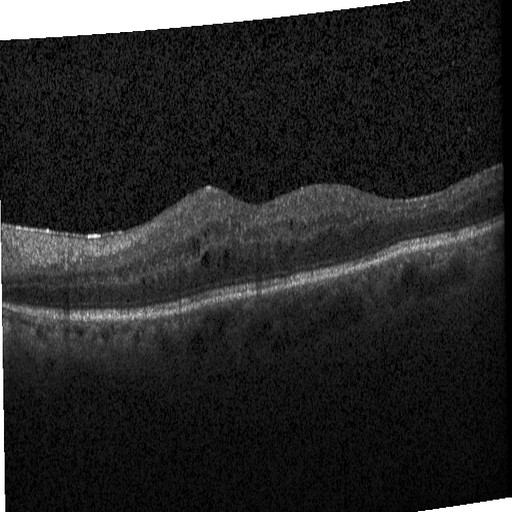
Macular OCT: diabetic macular edema.